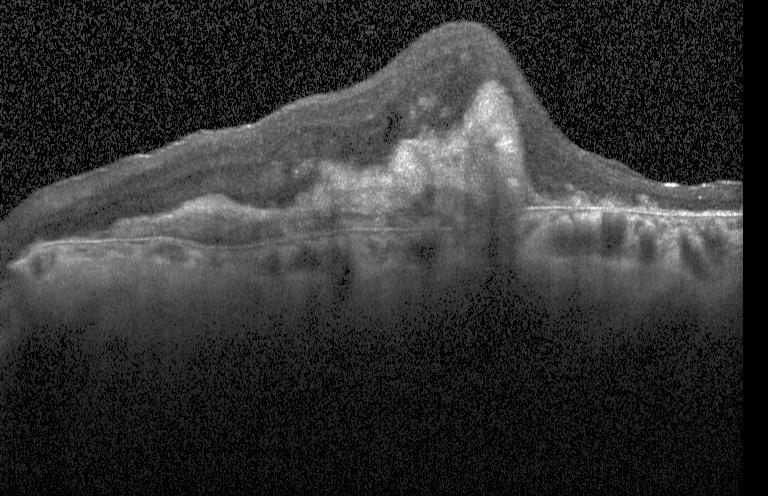 OCT finding: a choroidal neovascular membrane.